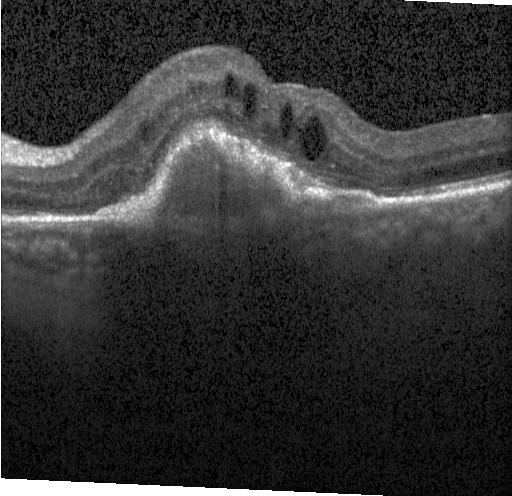
Finding: a choroidal neovascular membrane.